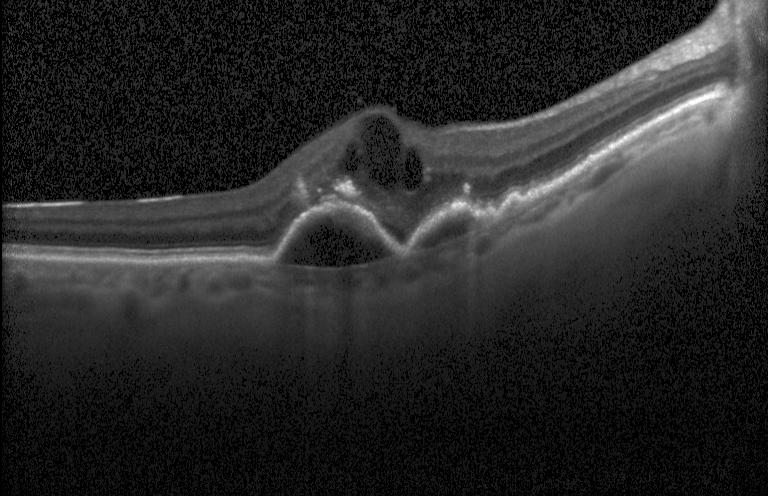 Impression: CNV.